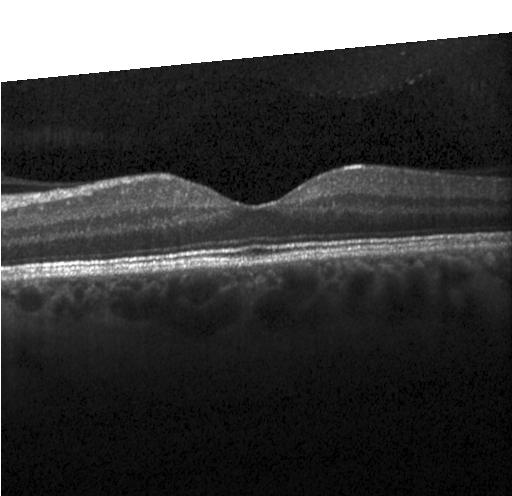
Finding: no choroidal neovascularization, diabetic macular edema, or drusen.